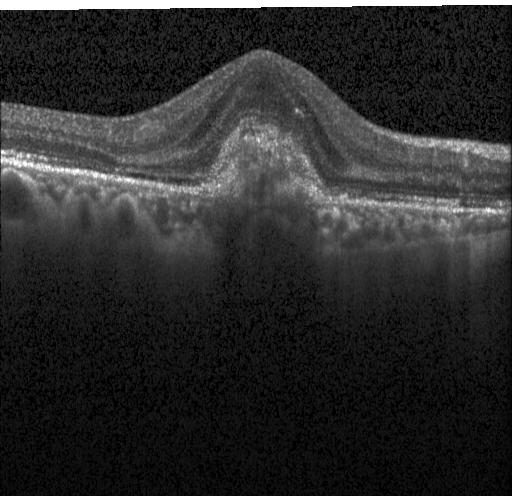
Through the macula. Retinal OCT cross-section. SD-OCT.
Dx: a choroidal neovascular membrane.